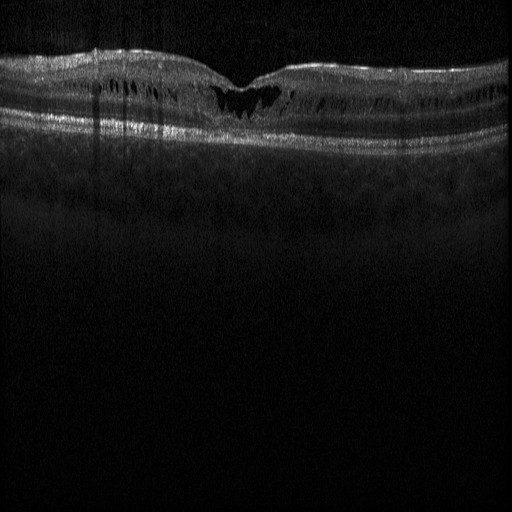

Heidelberg Spectralis; fovea-centered; SD-OCT; OCT B-scan — Impression: diabetic macular edema.